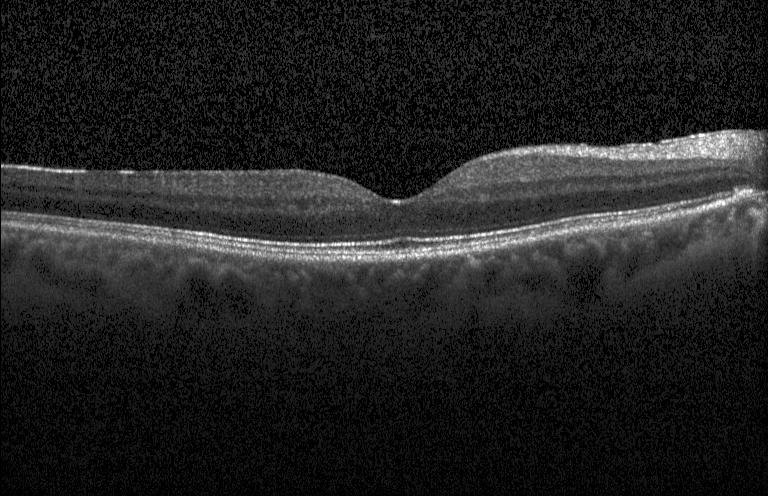
Instrument: Heidelberg Spectralis. OCT B-scan — Diagnosis: neither CNV, DME, nor drusen.